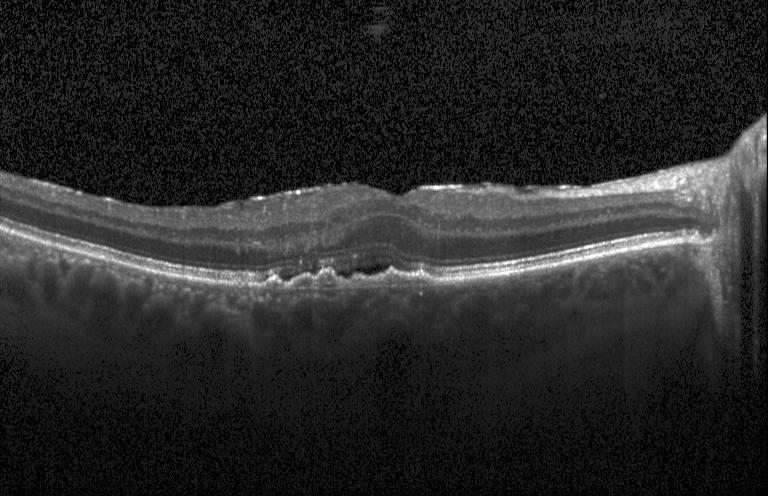
Instrument: Heidelberg Spectralis, OCT B-scan, spectral-domain optical coherence tomography. Impression: choroidal neovascularization.